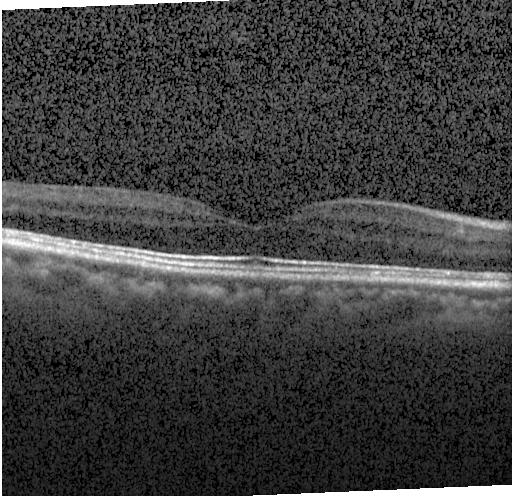 Retinal OCT cross-section — Neither choroidal neovascularization, diabetic macular edema, nor drusen.